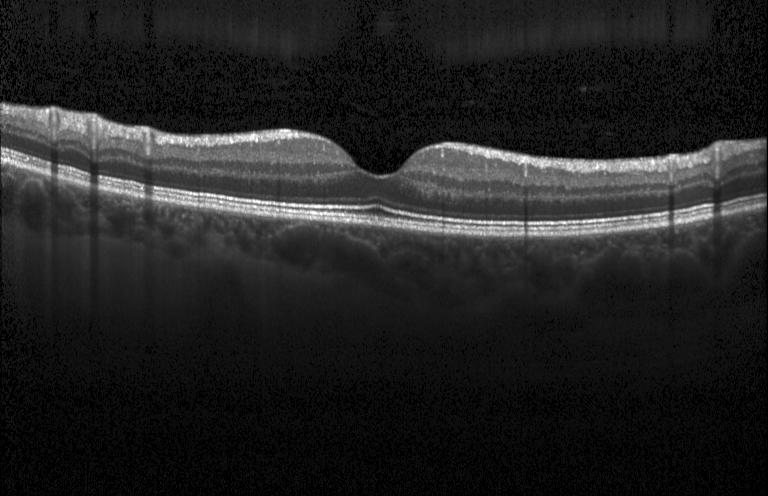 Diagnosis: no choroidal neovascularization, diabetic macular edema, or drusen.